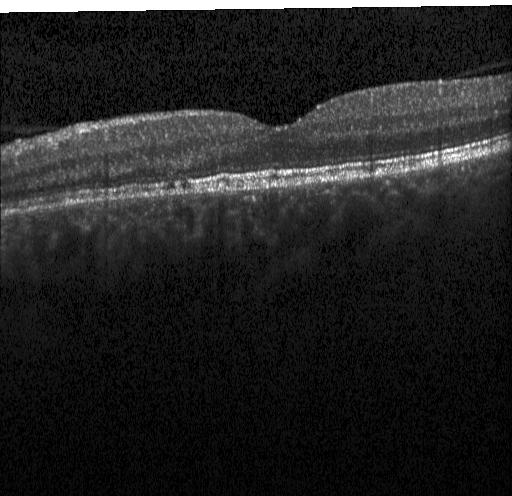

Centered on the fovea. OCT B-scan. Impression: no evidence of CNV, DME, or drusen.